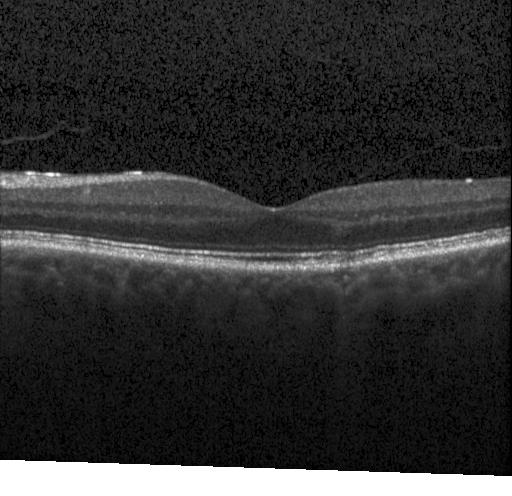
Diagnosis: no choroidal neovascularization, diabetic macular edema, or drusen.